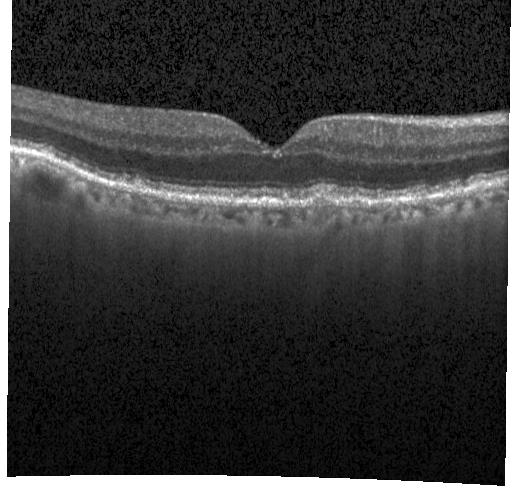
Retinal OCT B-scan.
Sub-RPE drusenoid deposits.